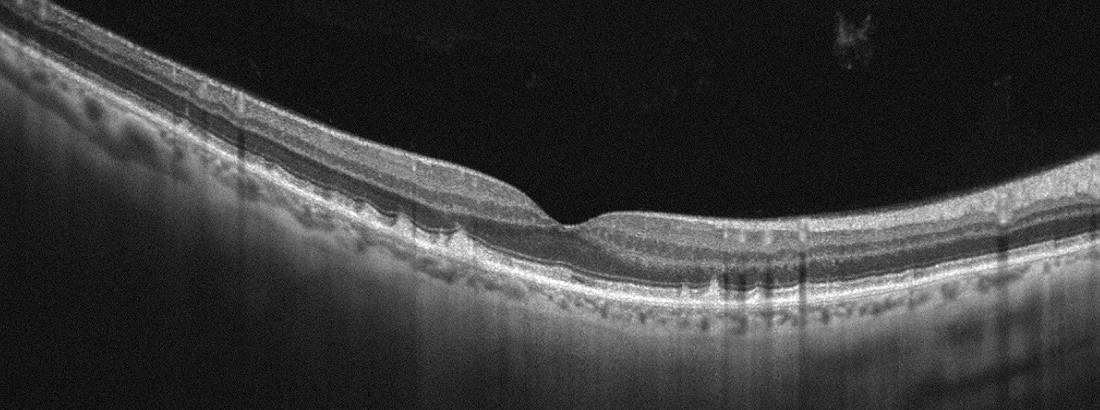 Through the macula, Optovue Avanti RTVue XR, OCT B-scan. The scan shows age-related macular degeneration (AMD).